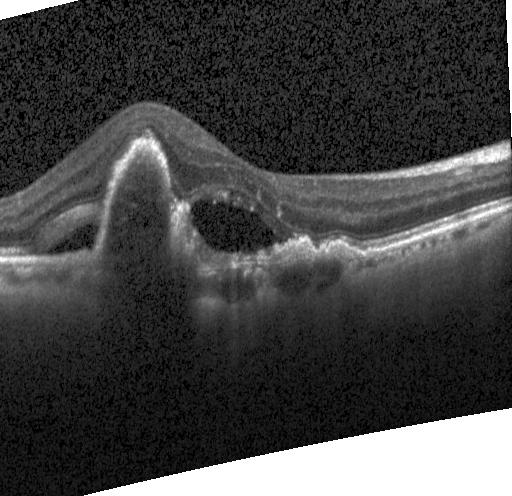
Impression: CNV.